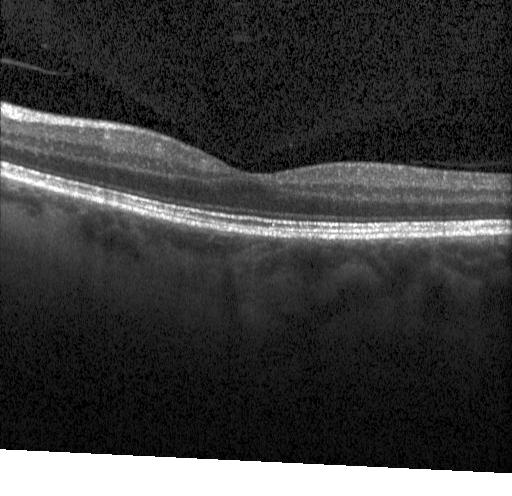 Through the macula. OCT B-scan — This B-scan demonstrates neither CNV, DME, nor drusen.